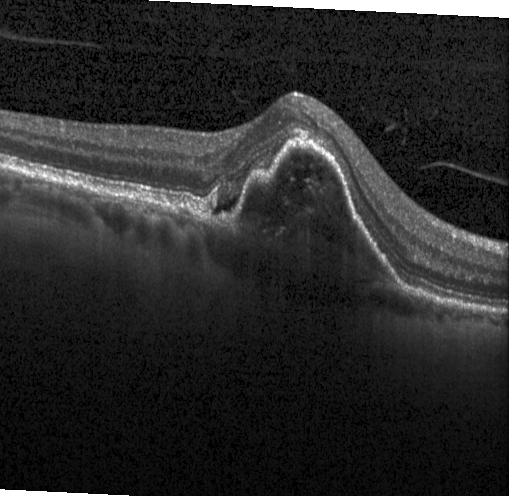
Centered on the fovea. Spectral-domain optical coherence tomography. Heidelberg Spectralis. Optical coherence tomography scan — Diagnosis: CNV.